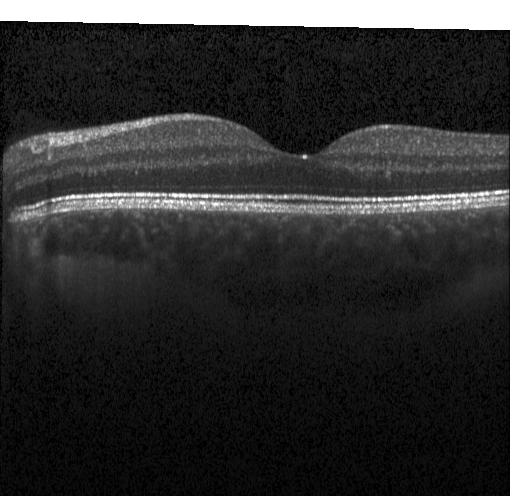 Spectral-domain OCT B-scan: no CNV, no DME, and no drusen.